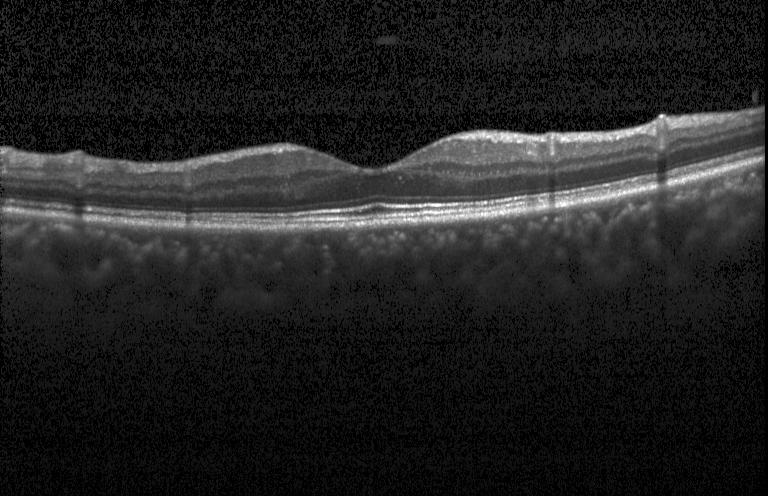 OCT B-scan, spectral-domain optical coherence tomography.
Finding: no choroidal neovascularization, diabetic macular edema, or drusen.